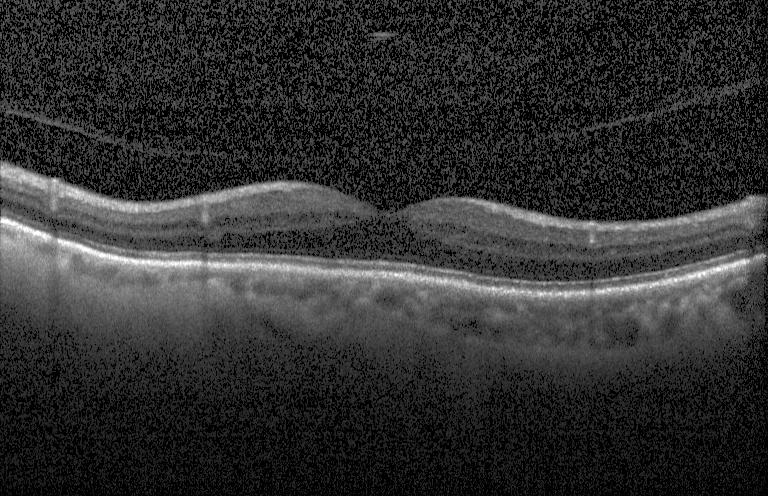

Optical coherence tomography scan, through the macula.
OCT finding: no choroidal neovascularization, diabetic macular edema, or drusen.